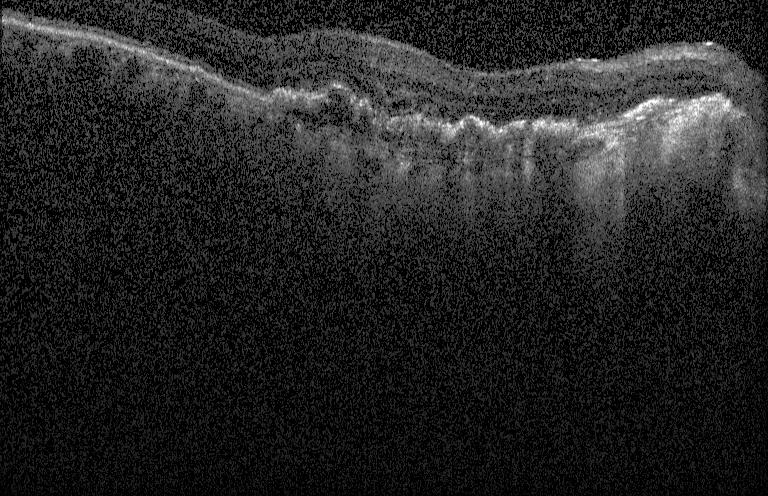 Macular OCT demonstrating a choroidal neovascular membrane.